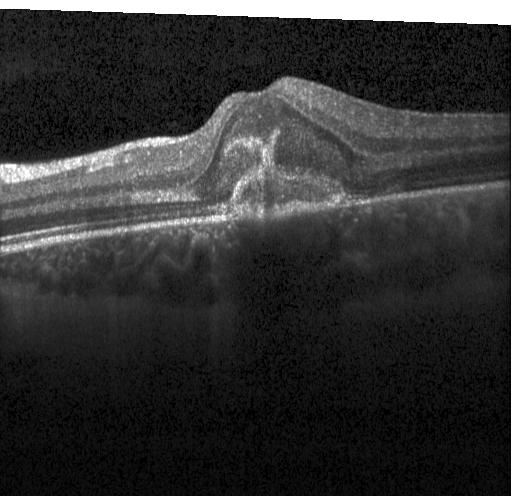

OCT finding: a choroidal neovascular membrane.